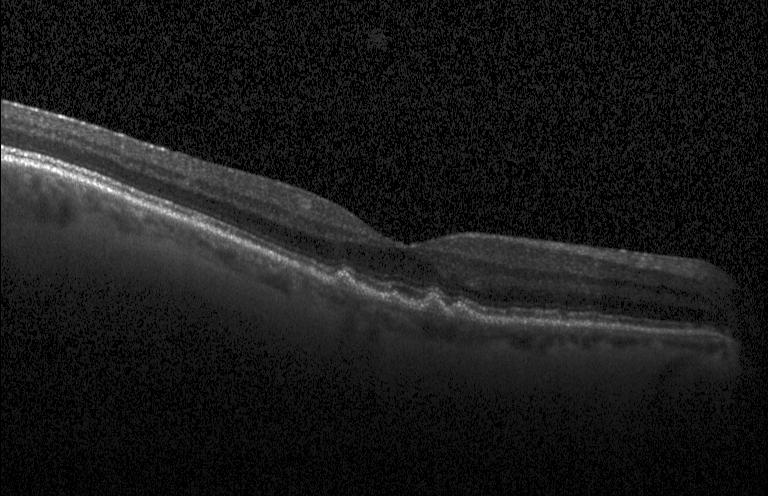

OCT B-scan, fovea-centered, instrument: Heidelberg Spectralis.
The scan shows drusen.